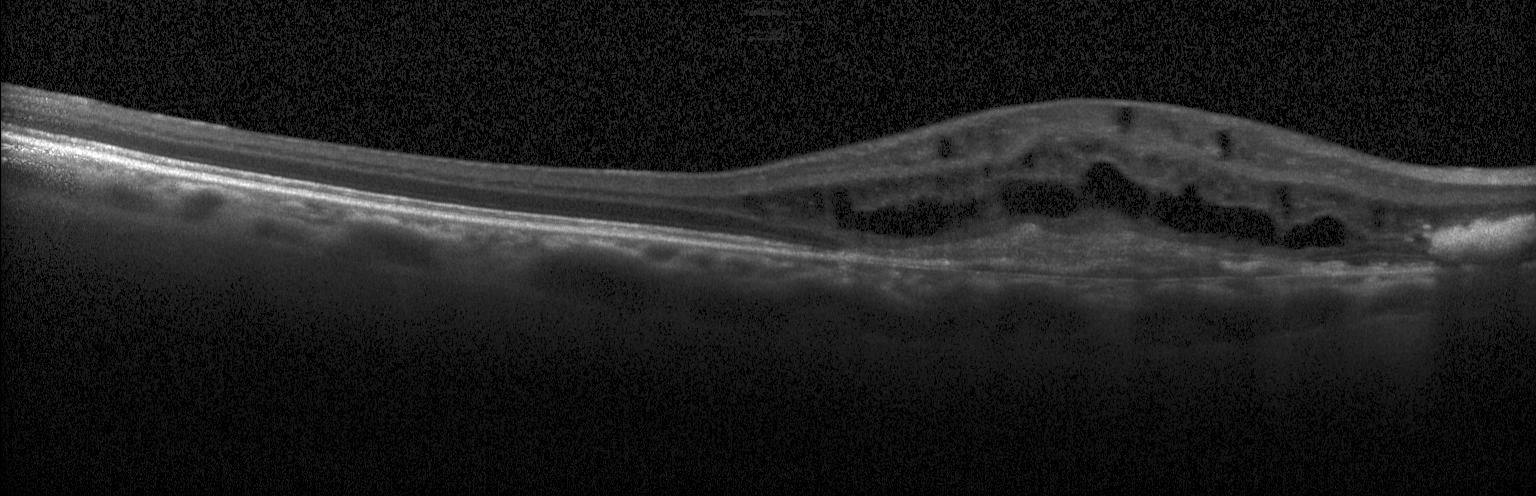 OCT finding: a choroidal neovascular membrane.